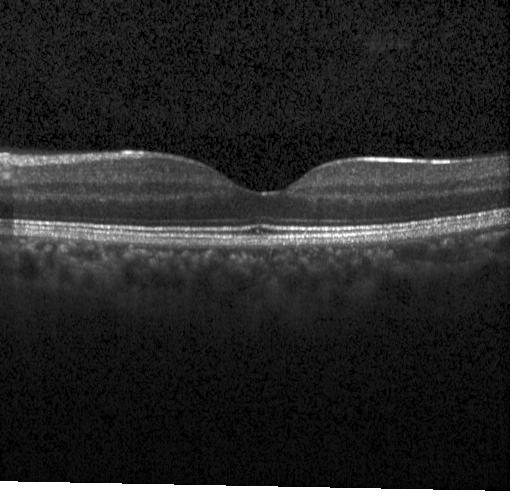 Retinal OCT cross-section showing no CNV, no DME, and no drusen.